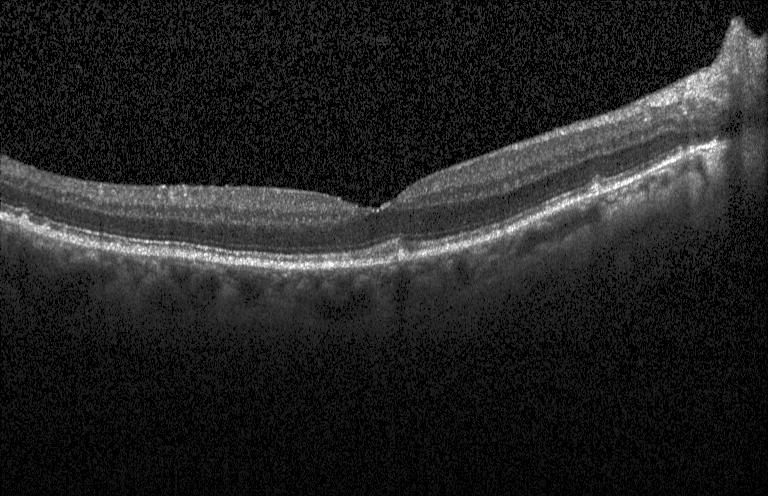

This B-scan demonstrates drusen.